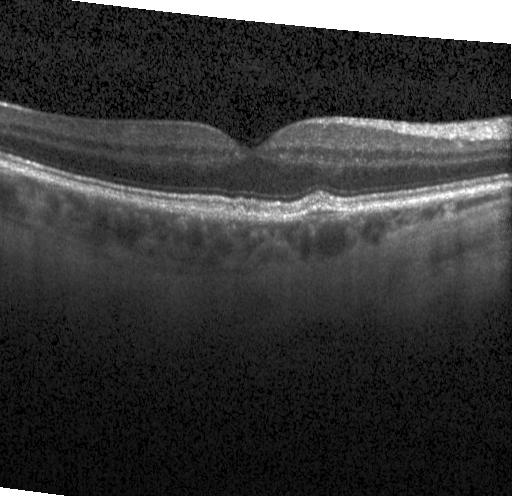
Diagnosis: sub-RPE drusenoid deposits.